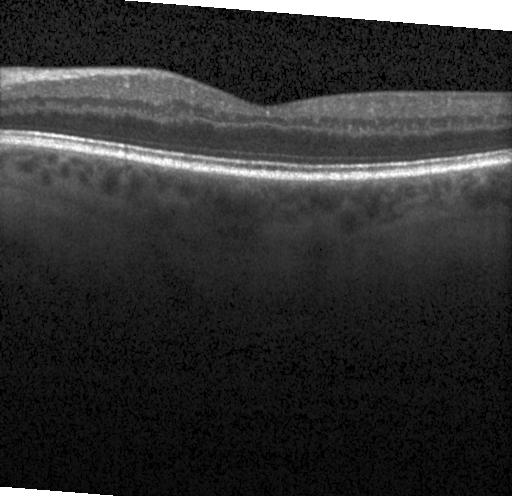

Heidelberg Spectralis, spectral-domain optical coherence tomography, optical coherence tomography B-scan — Impression: neither choroidal neovascularization, diabetic macular edema, nor drusen.